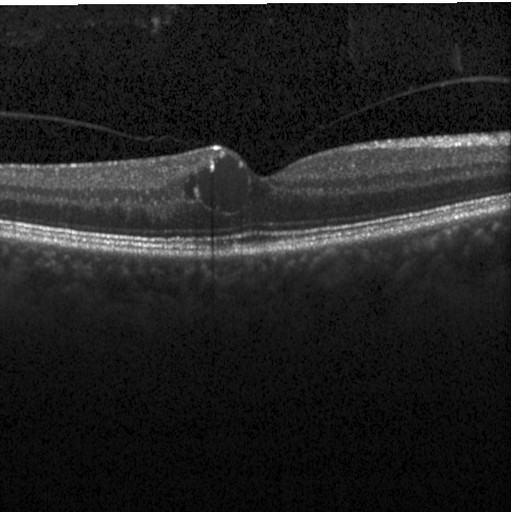
Retinal OCT cross-section. Assessment: diabetic macular edema (DME).